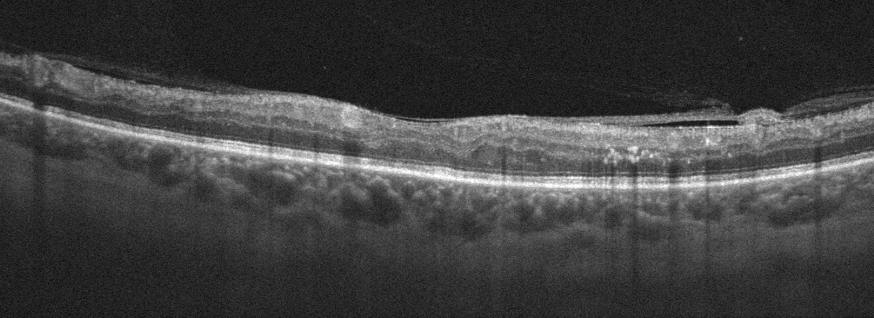

Optical coherence tomography B-scan; through the macula; Optovue Avanti RTVue XR. The scan shows diabetic macular edema (DME).